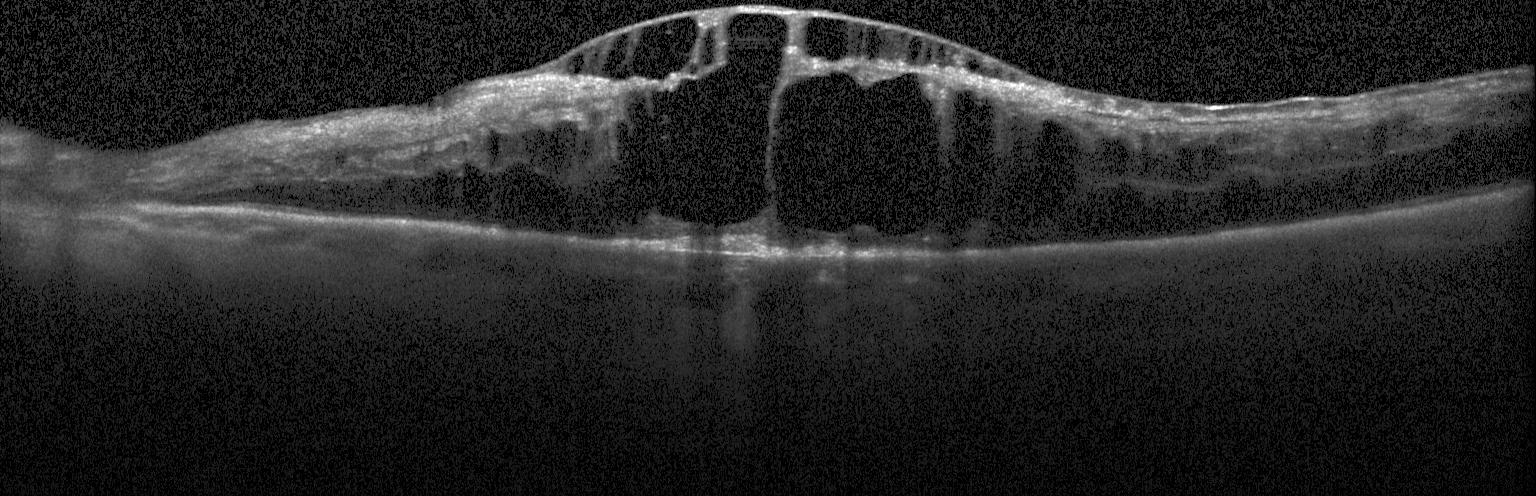

Diagnosis: diabetic macular edema.